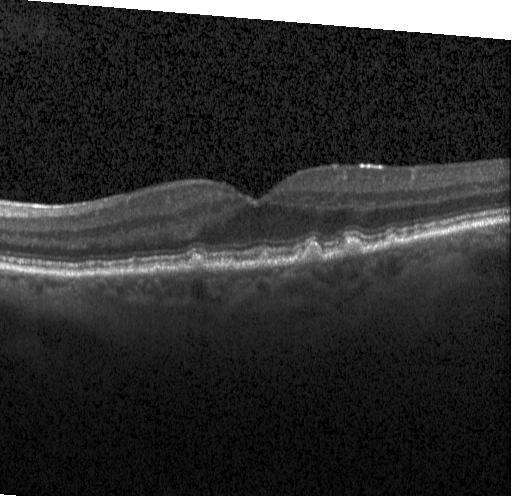
Impression: sub-RPE drusenoid deposits.